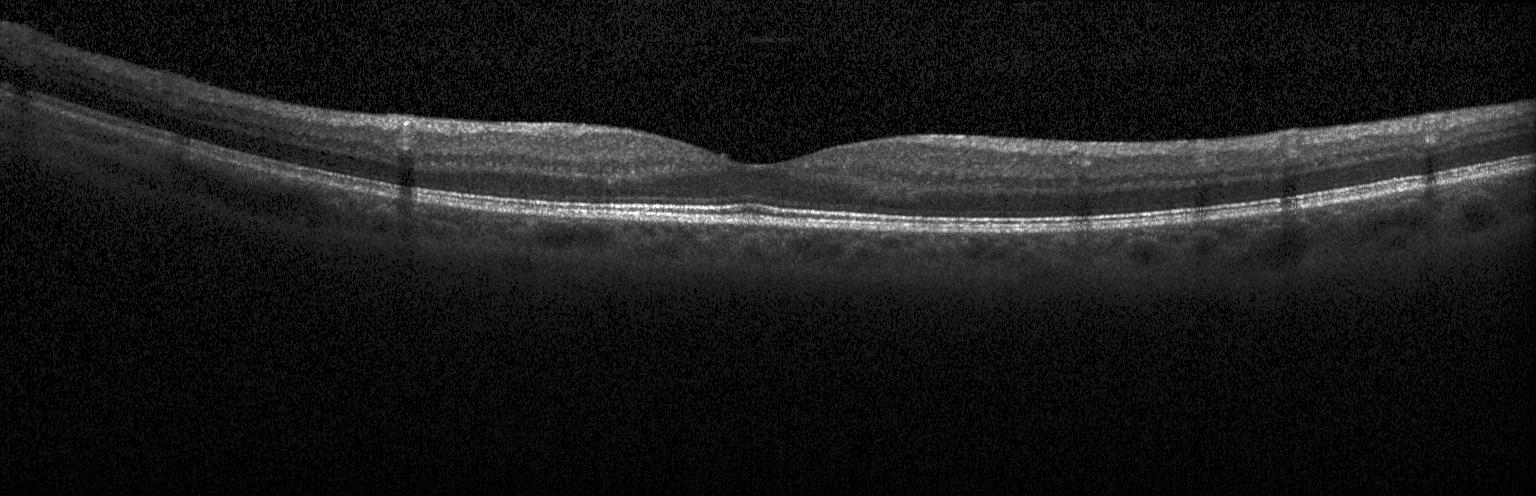
Spectral-domain OCT; retinal OCT B-scan; instrument: Heidelberg Spectralis — No CNV, no DME, and no drusen.